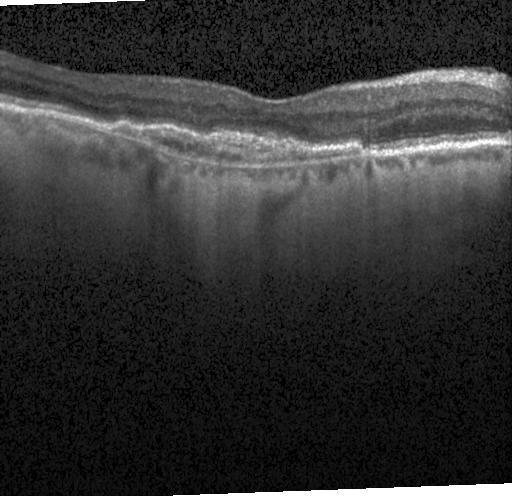

Horizontal scan through the fovea; OCT line scan — A choroidal neovascular membrane.